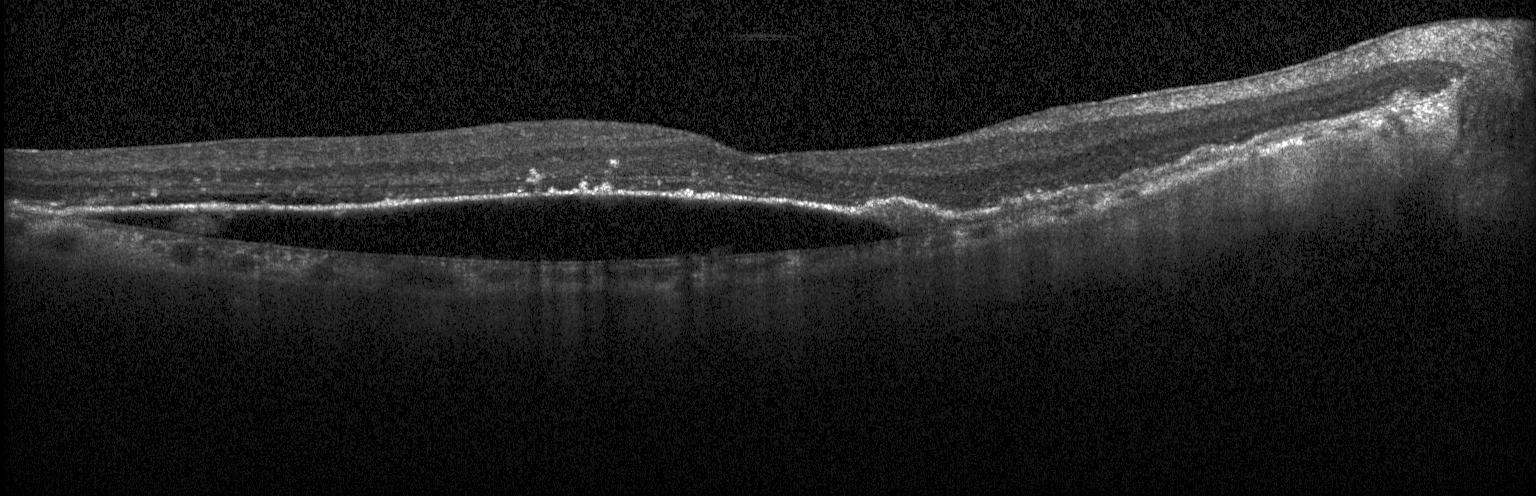

Impression: choroidal neovascularization (CNV).